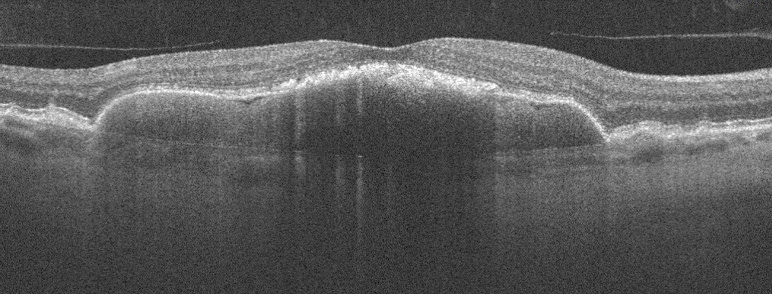
Through the macula; retinal OCT B-scan; instrument: Optovue Avanti RTVue XR.
Impression: AMD.